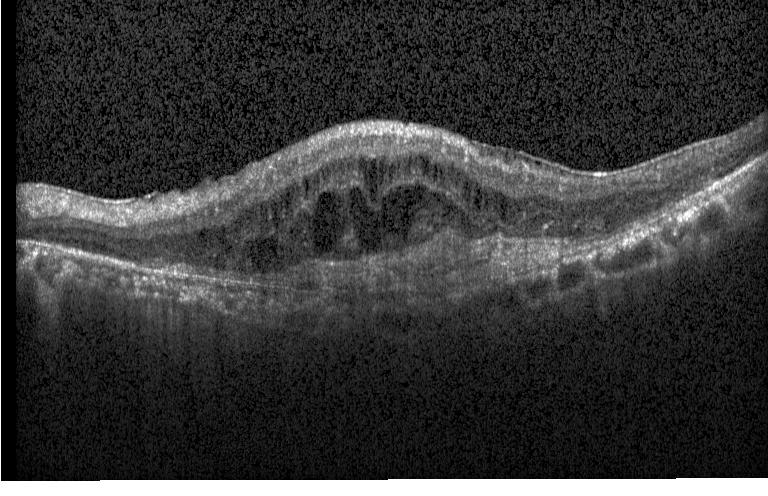 This B-scan demonstrates CNV.